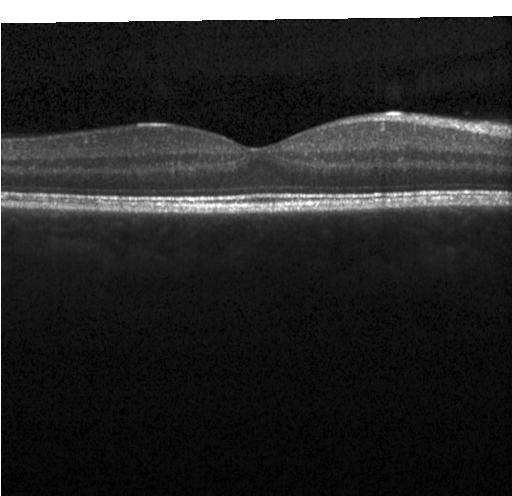 Impression: no choroidal neovascularization, diabetic macular edema, or drusen.